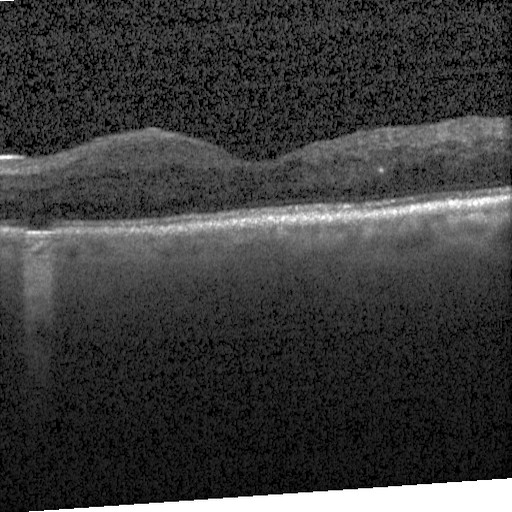

Retinal OCT cross-section; spectral-domain OCT.
This B-scan demonstrates diabetic macular edema (DME).